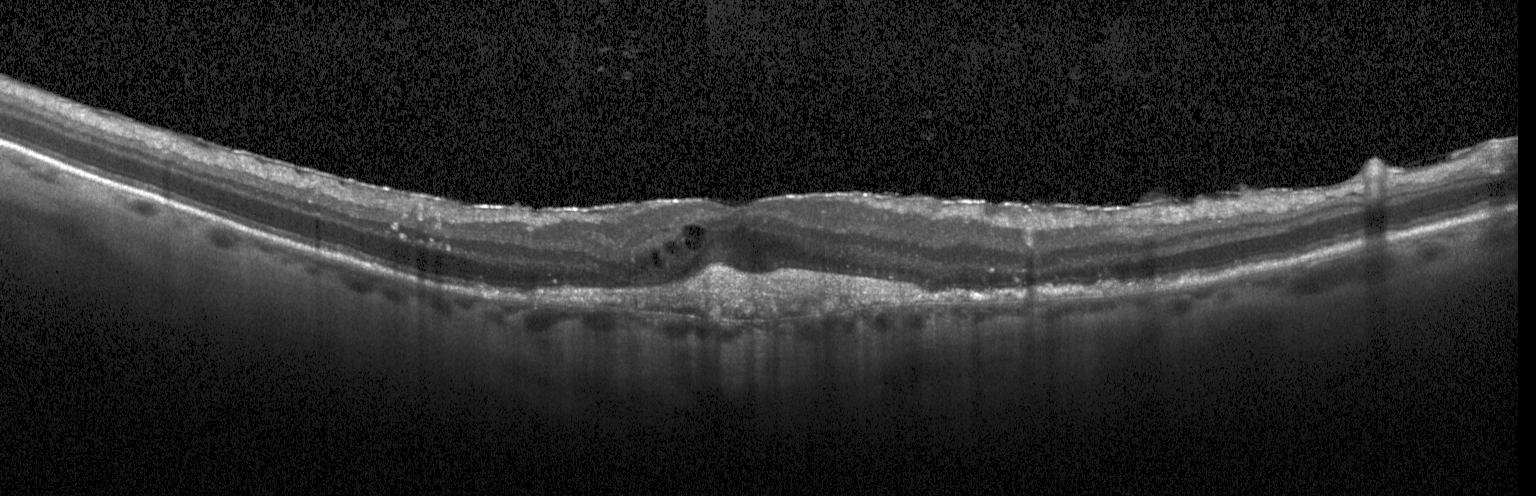
OCT finding: choroidal neovascularization (CNV).